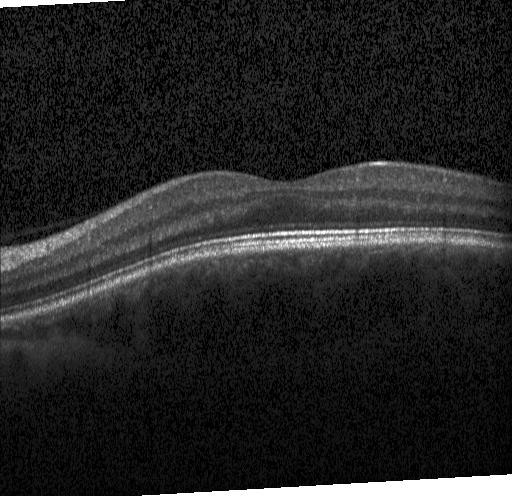

Heidelberg Spectralis · fovea-centered · optical coherence tomography B-scan · SD-OCT. Finding: neither CNV, DME, nor drusen.